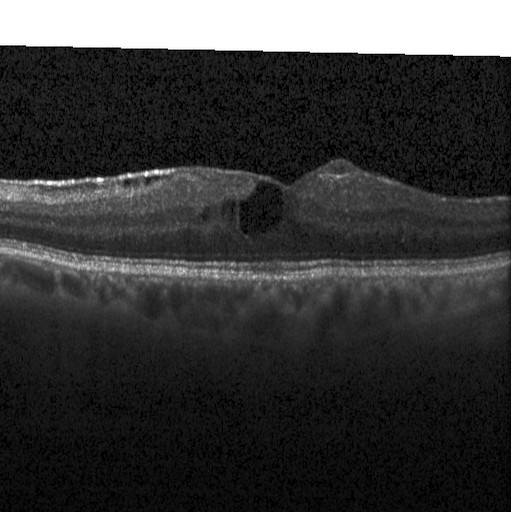

OCT line scan. Macular scan. Acquired on a Heidelberg Spectralis. Spectral-domain OCT — Impression: diabetic macular edema (DME).